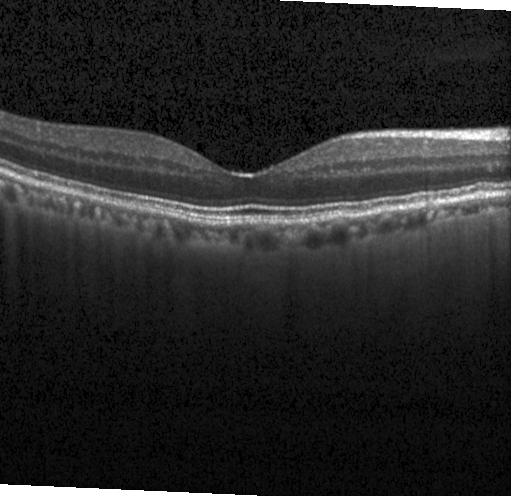

Diagnosis: no choroidal neovascularization, diabetic macular edema, or drusen.